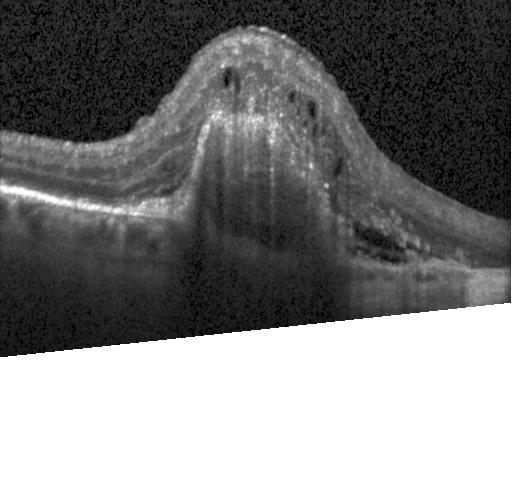
Retinal OCT cross-section
Impression: choroidal neovascularization (CNV).